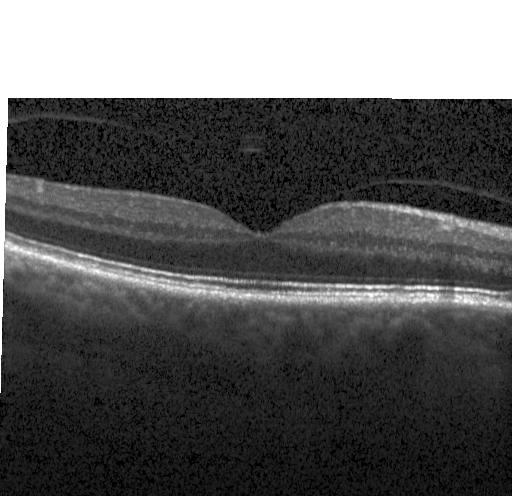
Finding: no evidence of choroidal neovascularization, diabetic macular edema, or drusen.